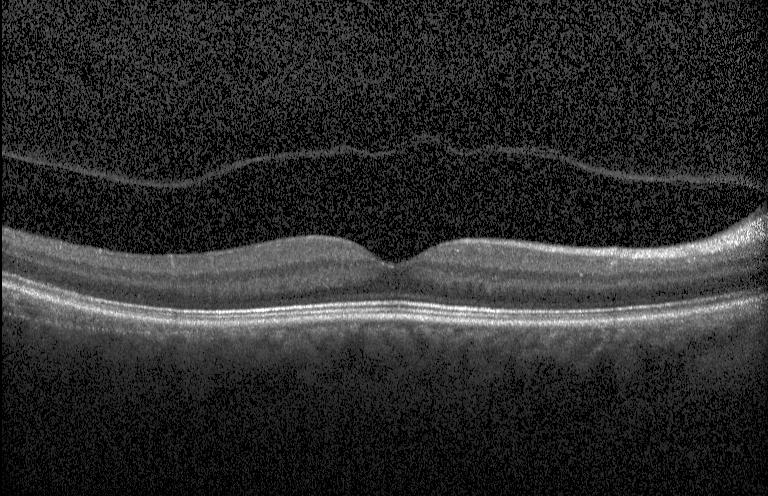 Macular OCT demonstrating neither choroidal neovascularization, diabetic macular edema, nor drusen.